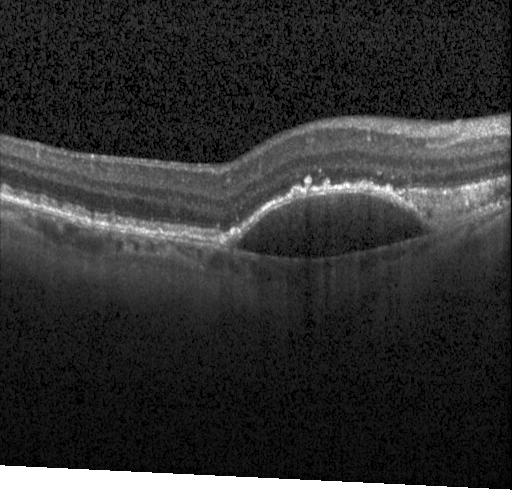
Retinal OCT B-scan. Instrument: Heidelberg Spectralis. SD-OCT. The scan shows CNV.